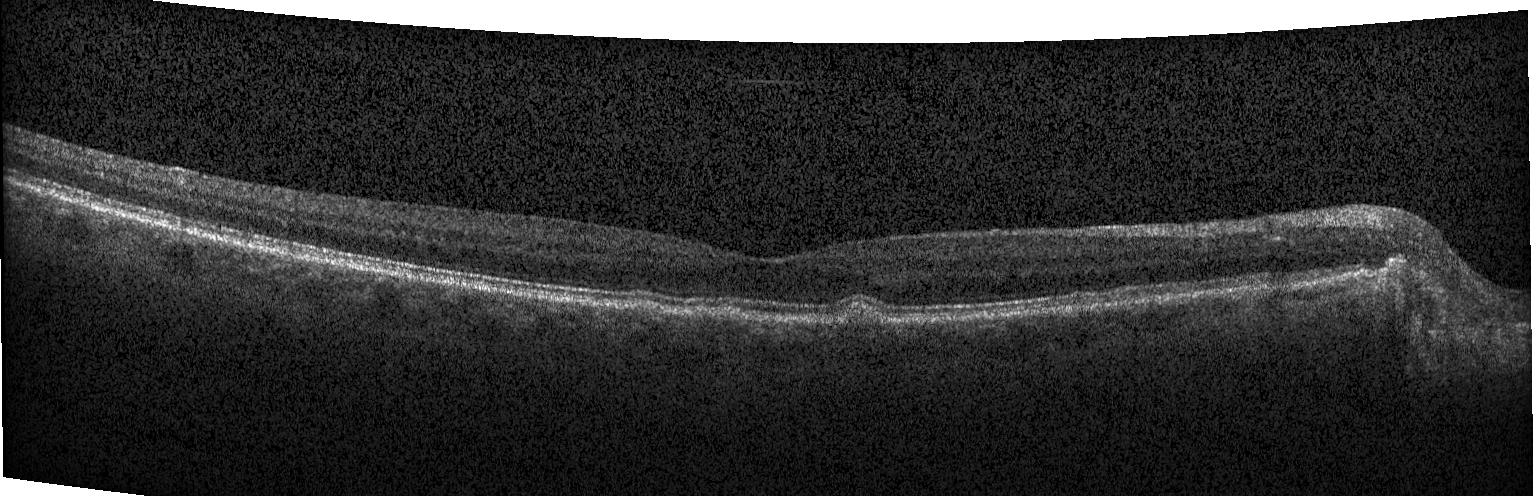
Spectral-domain OCT · centered on the fovea · OCT B-scan · Heidelberg Spectralis. Impression: multiple drusen.